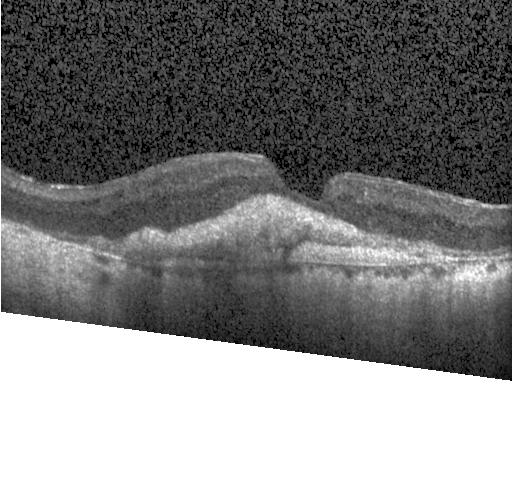

Spectral-domain OCT, retinal OCT B-scan. The scan shows a choroidal neovascular membrane.